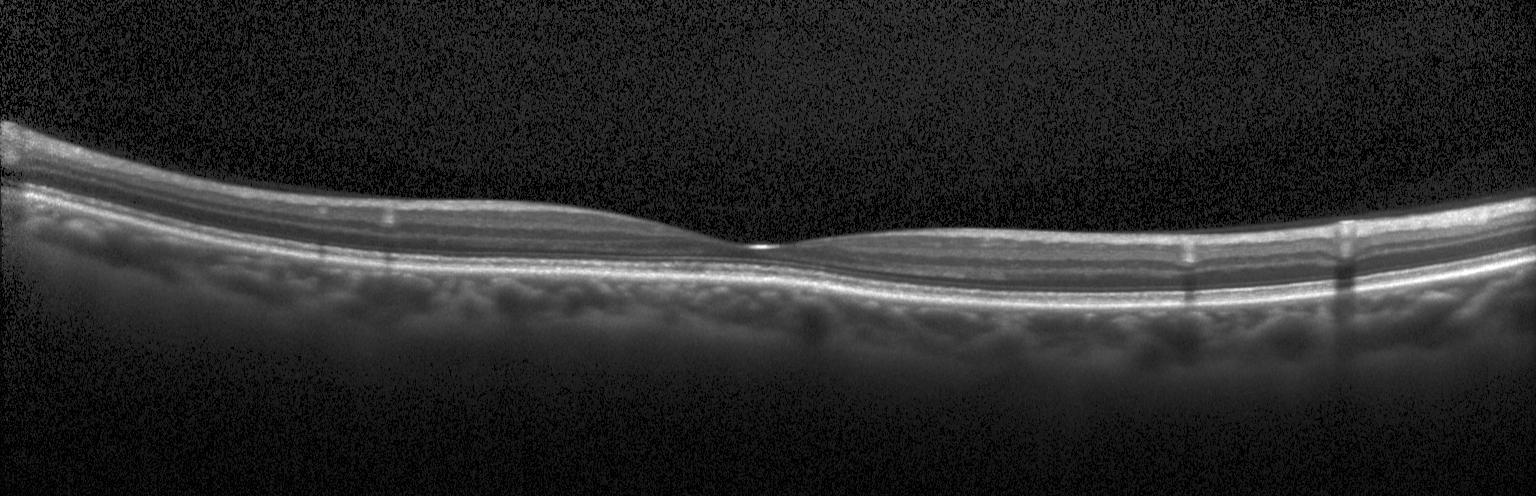 Diagnosis: no choroidal neovascularization, no diabetic macular edema, and no drusen.